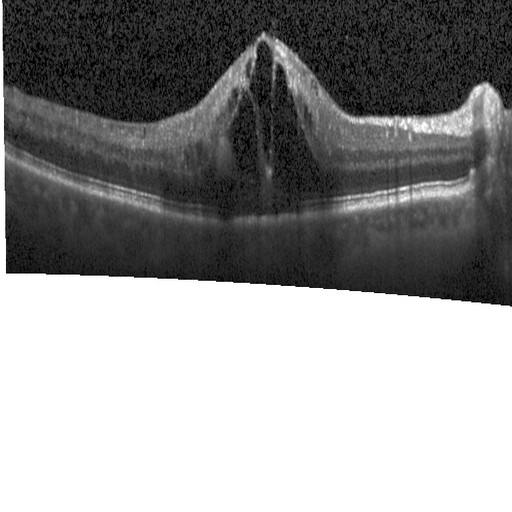
SD-OCT, optical coherence tomography scan, acquired on a Heidelberg Spectralis.
Finding: diabetic macular edema.